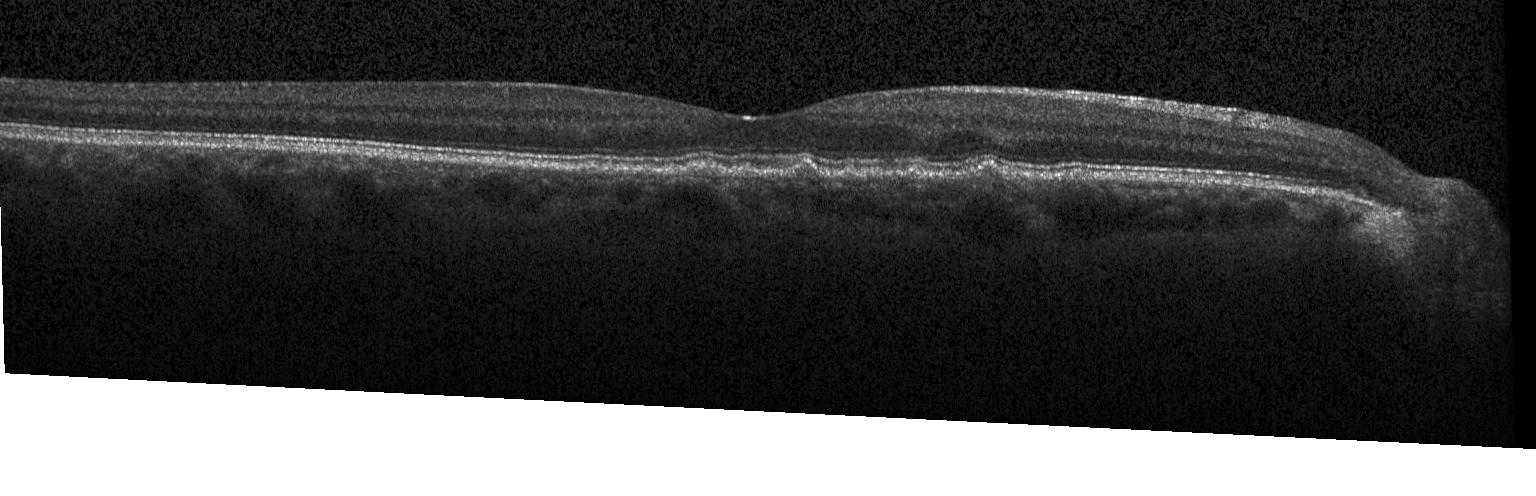

Macular scan, OCT line scan, Heidelberg Spectralis OCT system, spectral-domain OCT
This B-scan demonstrates drusen.